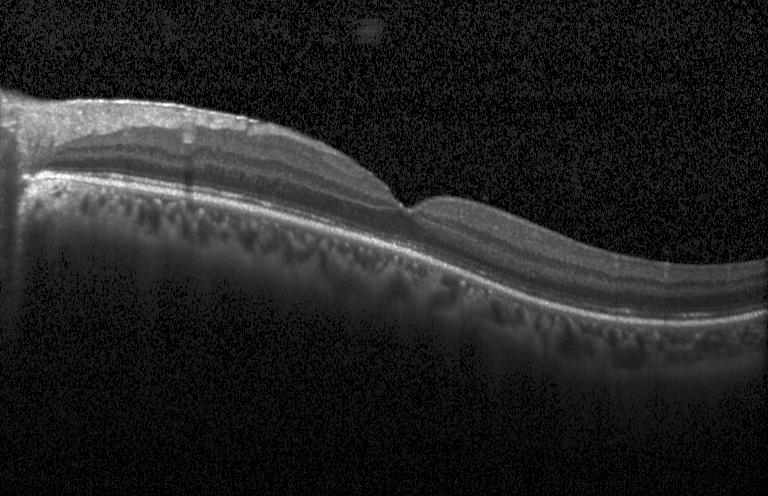 OCT line scan, through the macula — Diagnosis: neither choroidal neovascularization, diabetic macular edema, nor drusen.